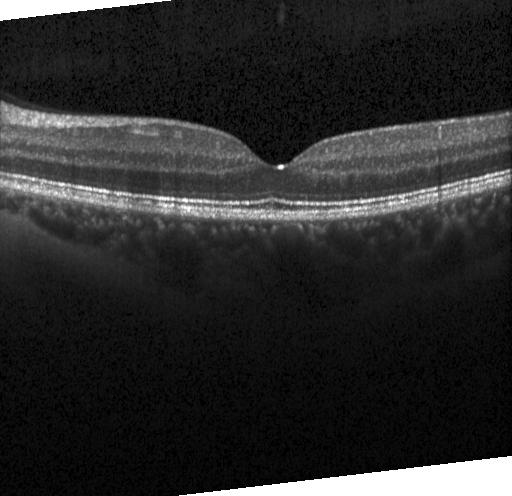 Optical coherence tomography B-scan.
No choroidal neovascularization, no diabetic macular edema, and no drusen.